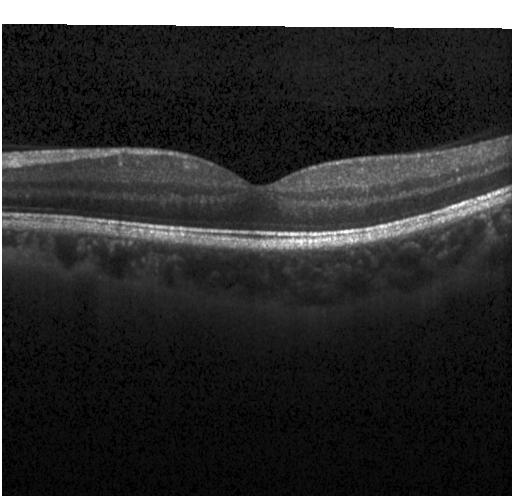 Heidelberg Spectralis OCT system · SD-OCT · retinal OCT cross-section
Impression: neither choroidal neovascularization, diabetic macular edema, nor drusen.